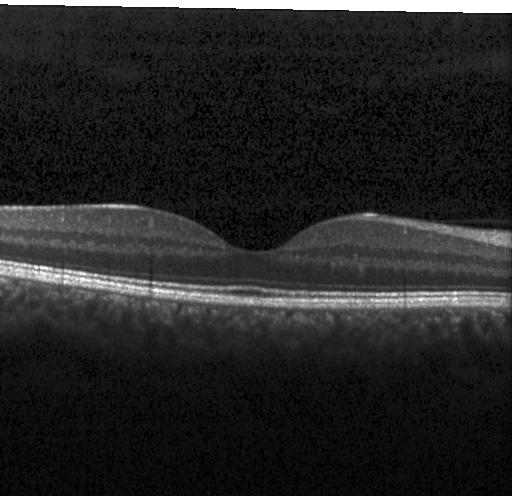

Spectral-domain optical coherence tomography. OCT line scan
Finding: neither choroidal neovascularization, diabetic macular edema, nor drusen.